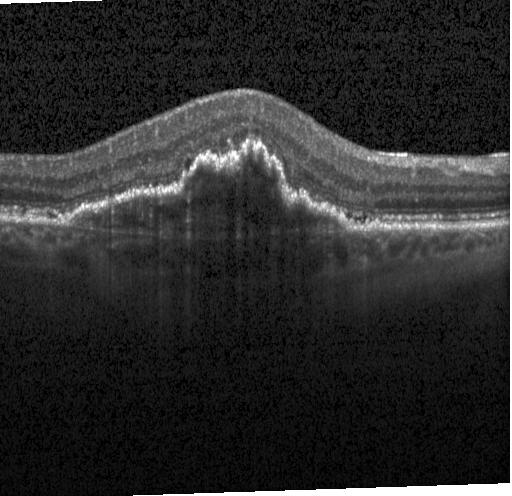

Macular OCT: choroidal neovascularization.